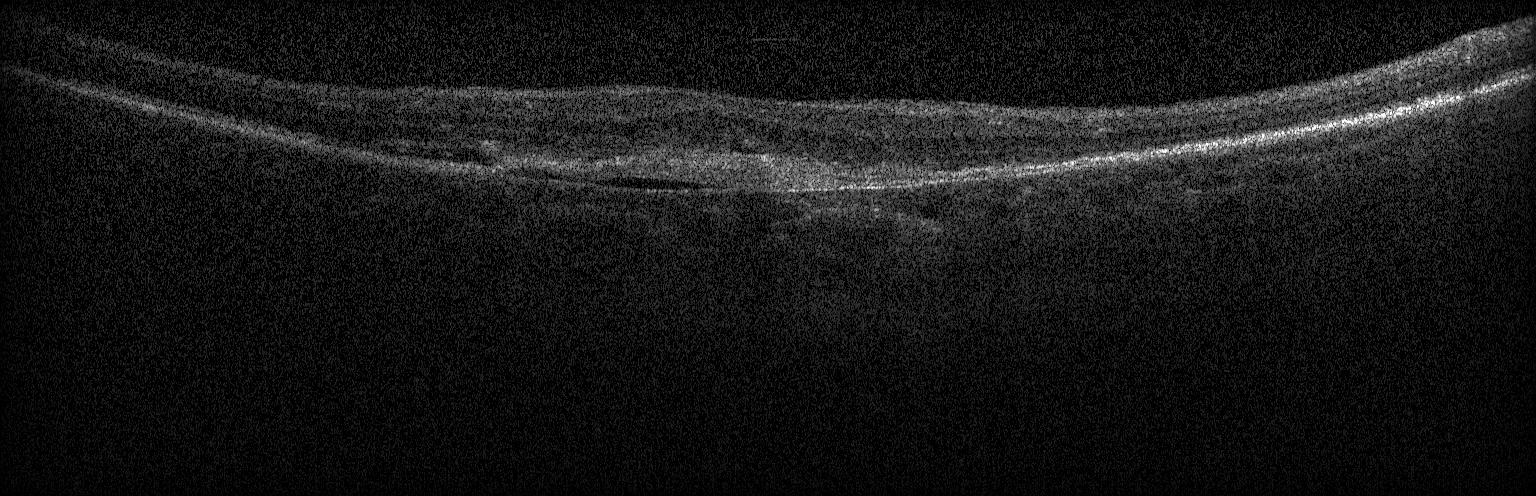
Spectral-domain OCT; instrument: Heidelberg Spectralis; optical coherence tomography B-scan; horizontal scan through the fovea — Assessment: choroidal neovascularization.